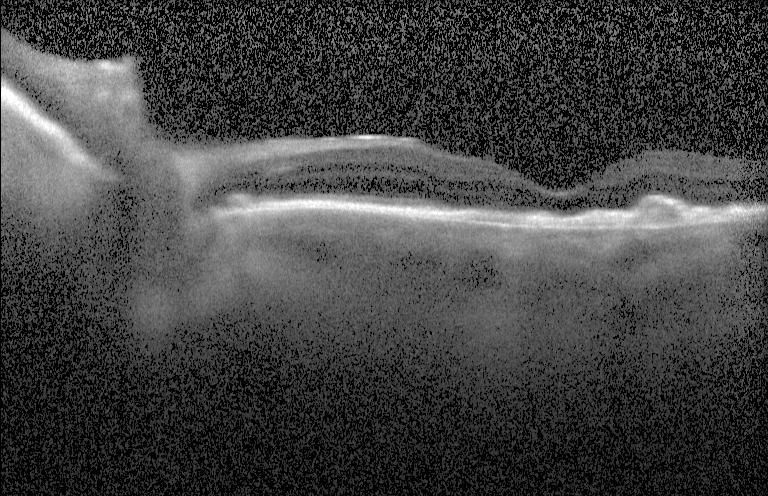
OCT line scan, spectral-domain optical coherence tomography. Dx: choroidal neovascularization.